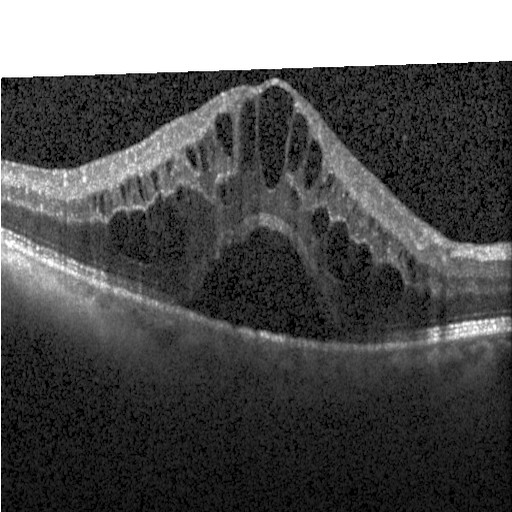 Optical coherence tomography scan. Finding: DME.